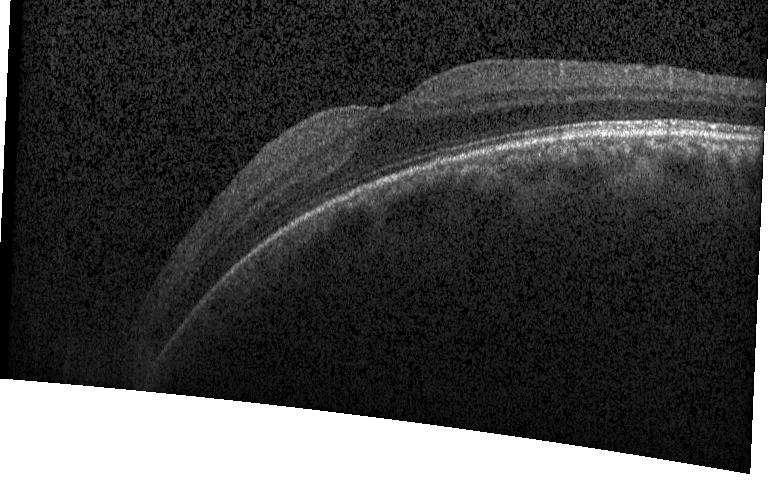

Spectral-domain optical coherence tomography, fovea-centered, retinal OCT B-scan, Heidelberg Spectralis OCT system.
Impression: no CNV, DME, or drusen.